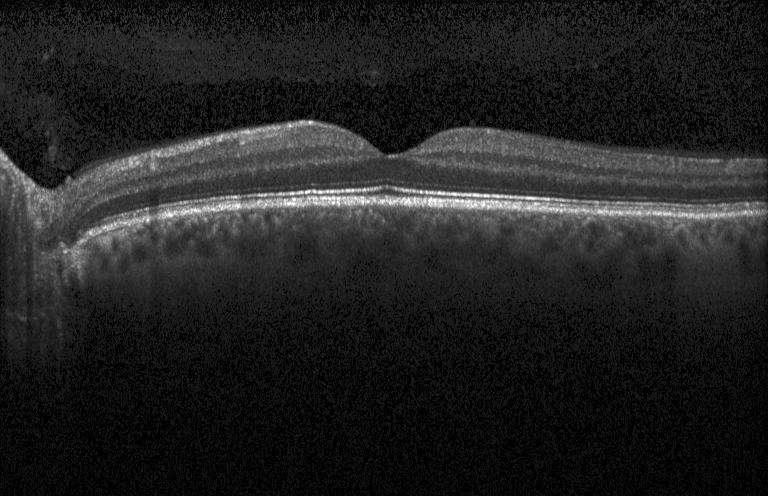 Finding: no CNV, no DME, and no drusen.